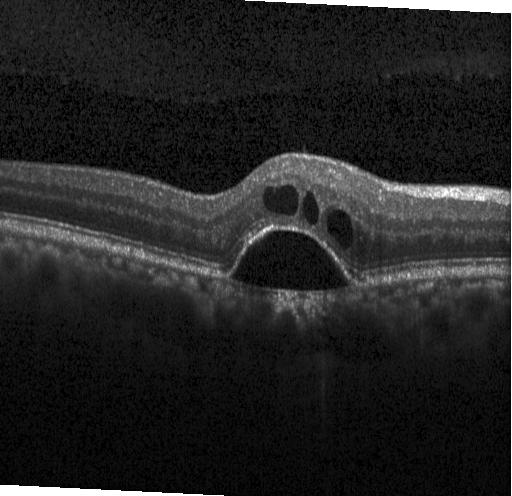 OCT scan showing a choroidal neovascular membrane.